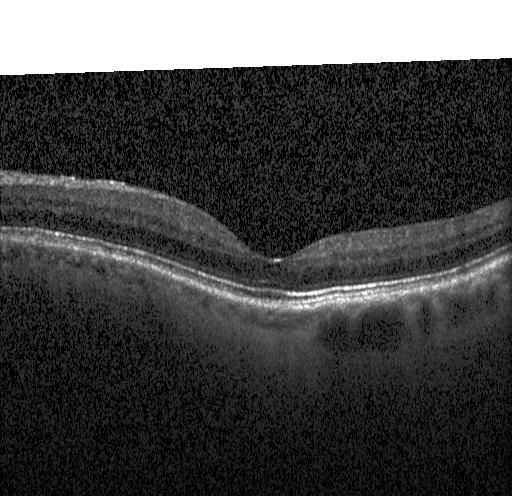 Acquired on a Heidelberg Spectralis. OCT line scan. Macular scan. SD-OCT.
Macular OCT: neither choroidal neovascularization, diabetic macular edema, nor drusen.